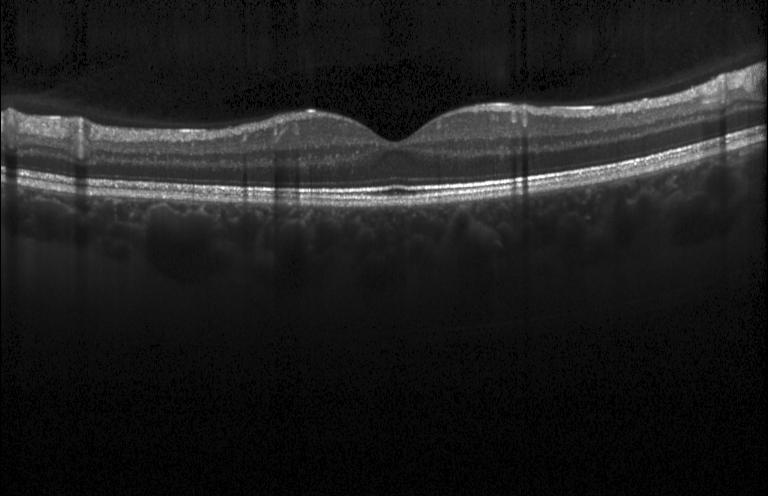 Finding: no CNV, no DME, and no drusen.